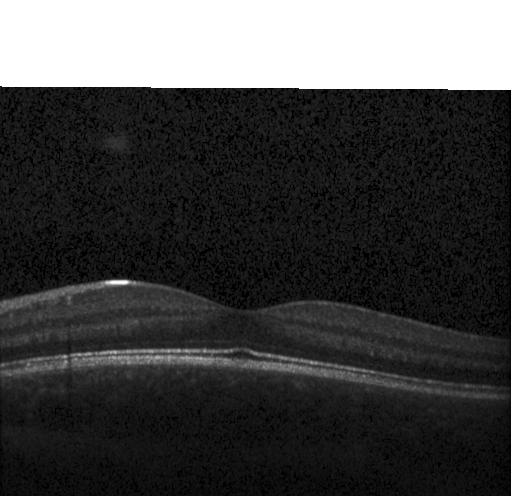 Optical coherence tomography B-scan. OCT finding: no evidence of choroidal neovascularization, diabetic macular edema, or drusen.